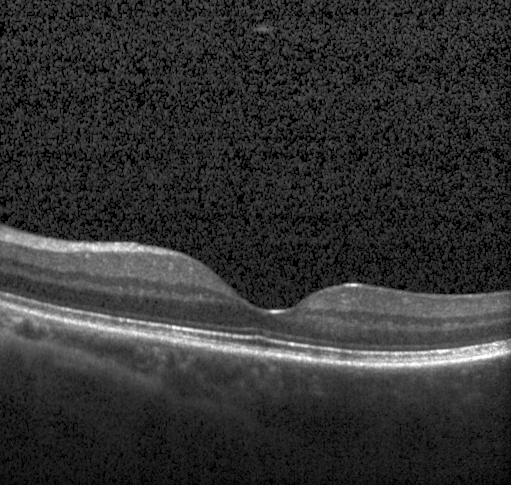 Retinal OCT B-scan.
Assessment: no evidence of choroidal neovascularization, diabetic macular edema, or drusen.